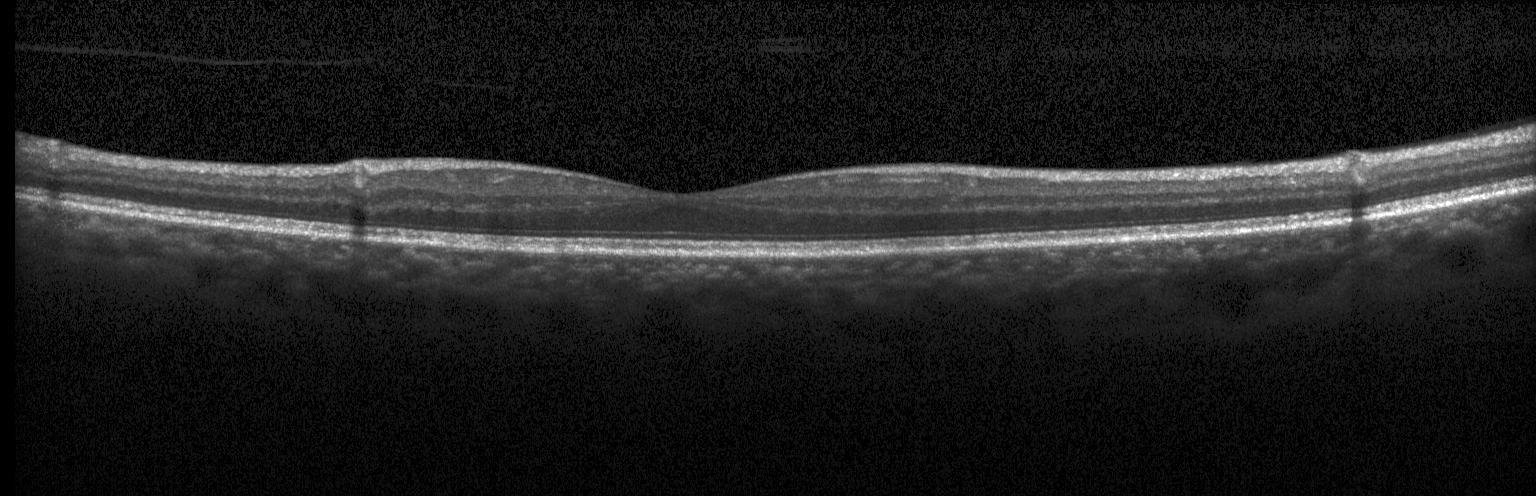

OCT B-scan. SD-OCT. Horizontal scan through the fovea — Assessment: neither choroidal neovascularization, diabetic macular edema, nor drusen.